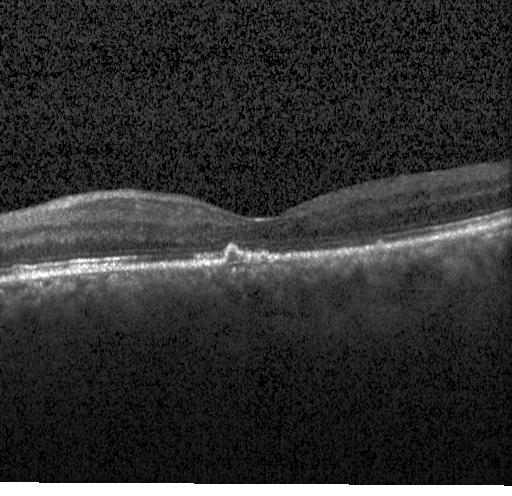

Assessment: drusen.